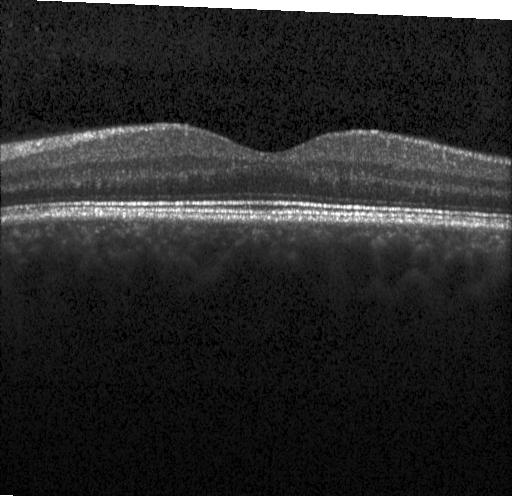

OCT line scan; SD-OCT.
Diagnosis: no evidence of CNV, DME, or drusen.